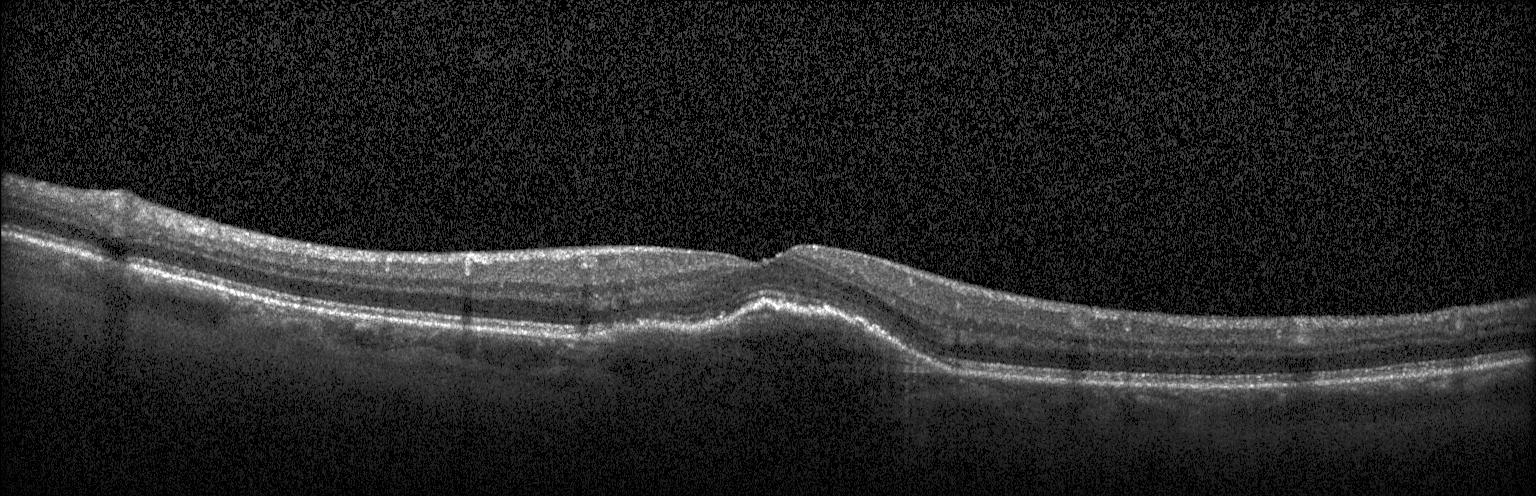

Optical coherence tomography scan · acquired on a Heidelberg Spectralis. Impression: a choroidal neovascular membrane.